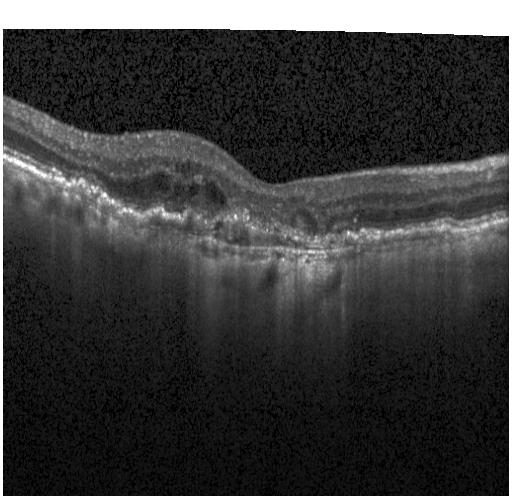

Spectral-domain OCT; optical coherence tomography scan
OCT finding: CNV.